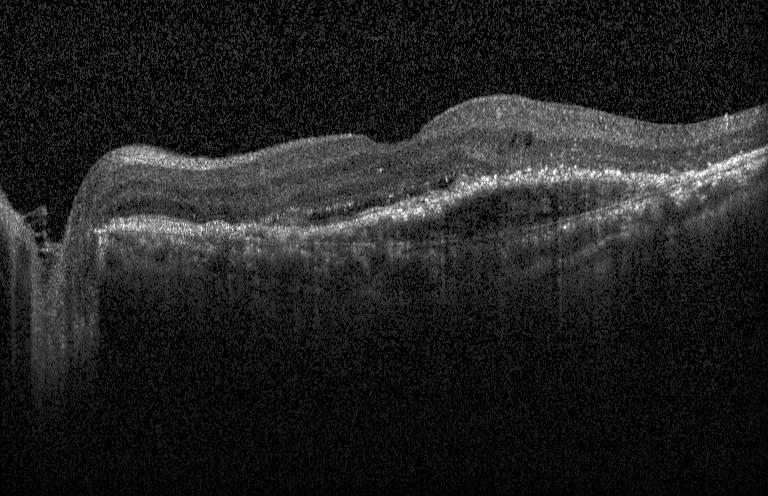 Spectral-domain optical coherence tomography; optical coherence tomography scan.
OCT finding: a choroidal neovascular membrane.